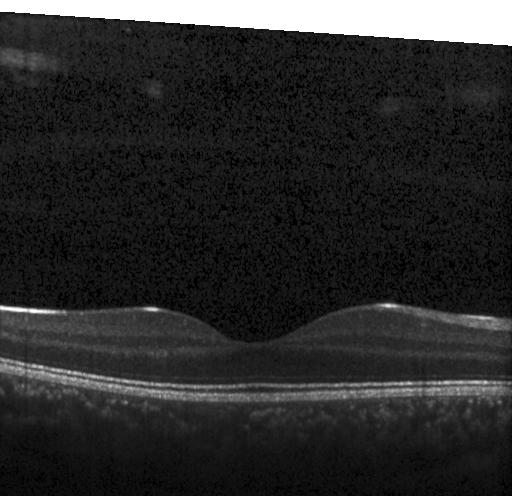
Retinal OCT cross-section — Finding: no choroidal neovascularization, no diabetic macular edema, and no drusen.